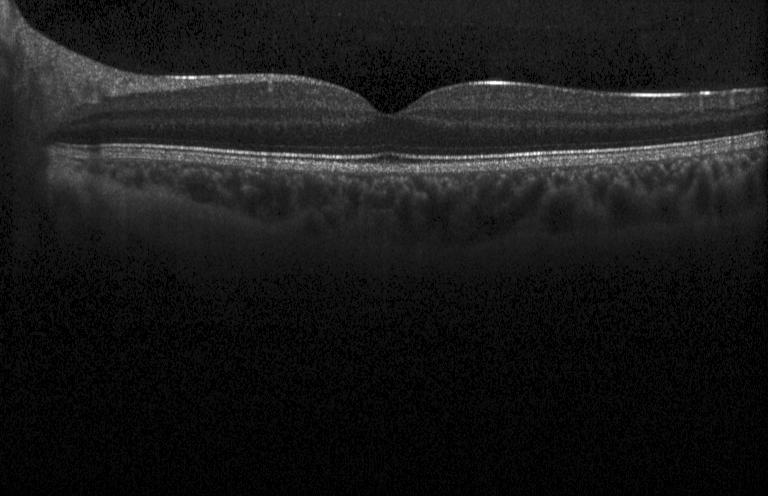 Acquired on a Heidelberg Spectralis; OCT B-scan. This B-scan demonstrates no CNV, no DME, and no drusen.